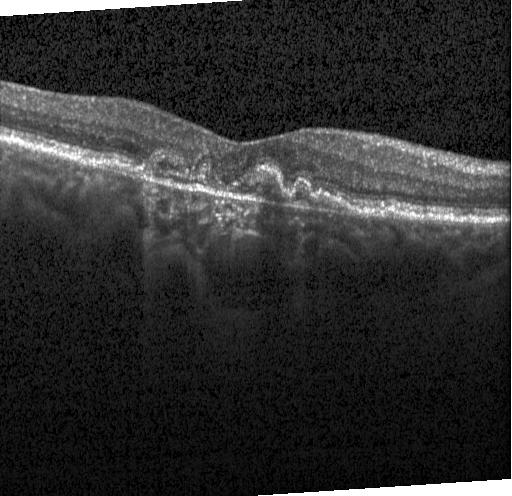

Diagnosis: choroidal neovascularization.